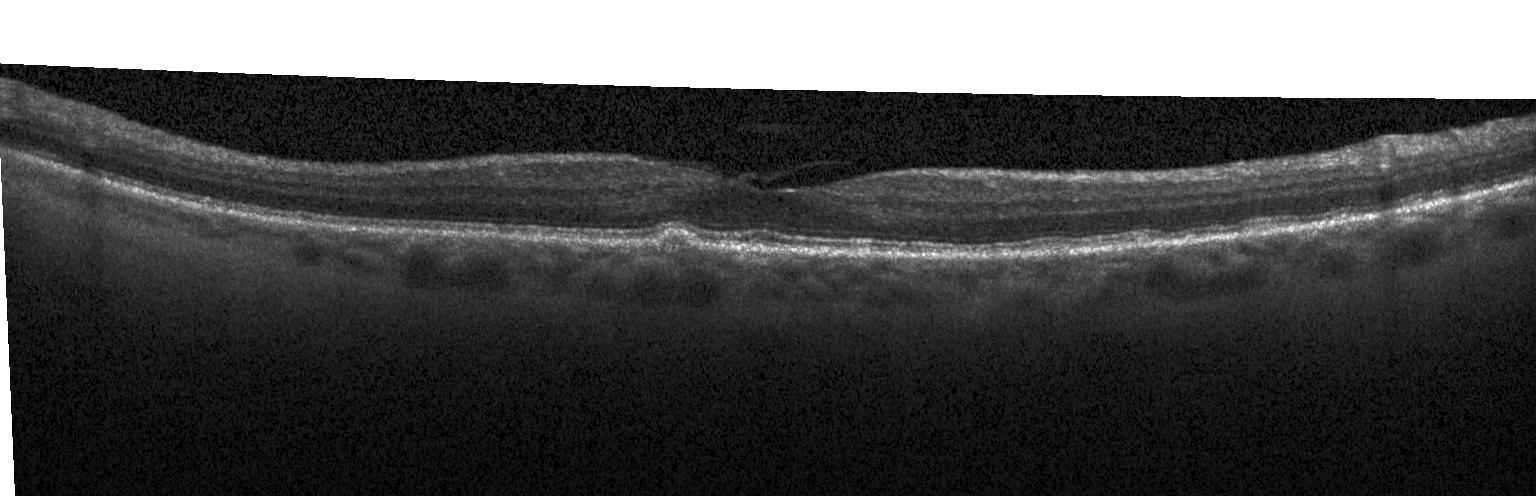
Retinal OCT cross-section. The scan shows drusen.